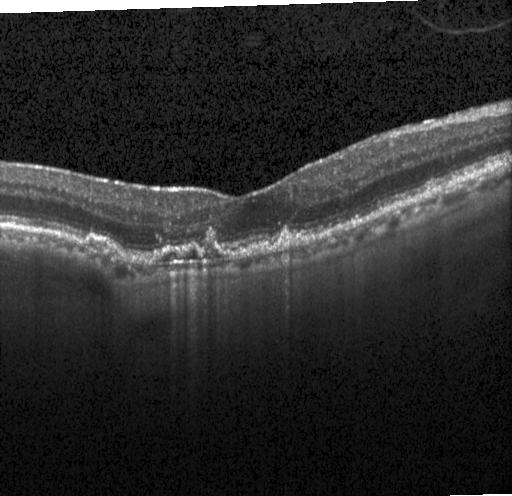
Horizontal scan through the fovea; Heidelberg Spectralis; SD-OCT; retinal OCT cross-section. Finding: a choroidal neovascular membrane.